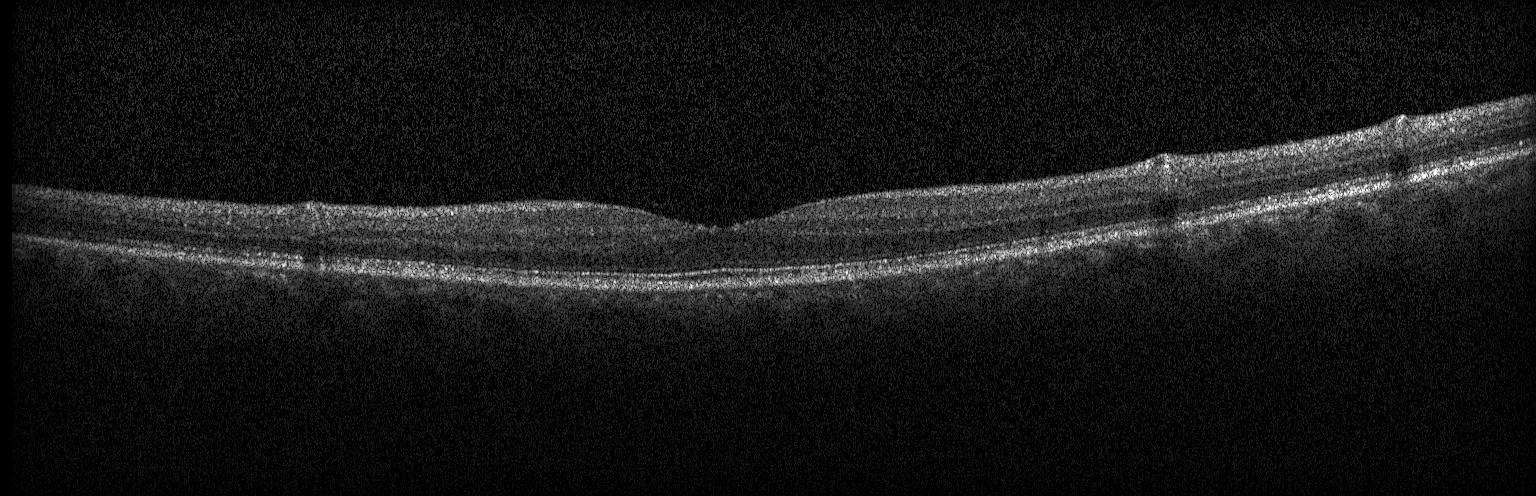

Retinal OCT B-scan; spectral-domain optical coherence tomography; instrument: Heidelberg Spectralis; centered on the fovea — No choroidal neovascularization, no diabetic macular edema, and no drusen.